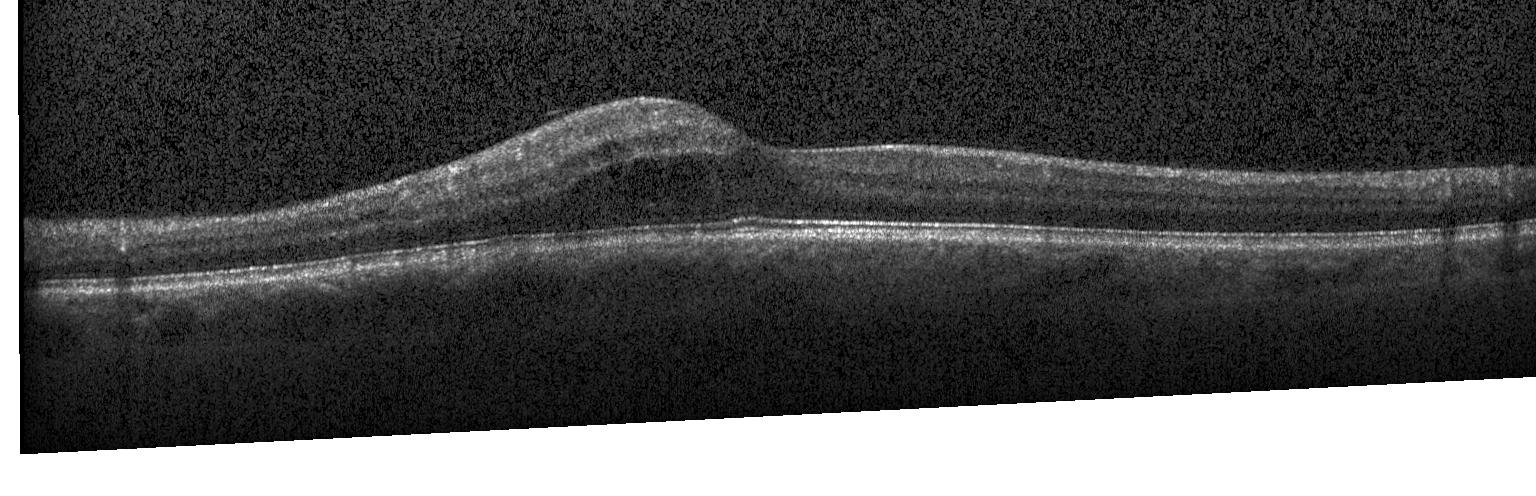 Dx: DME.